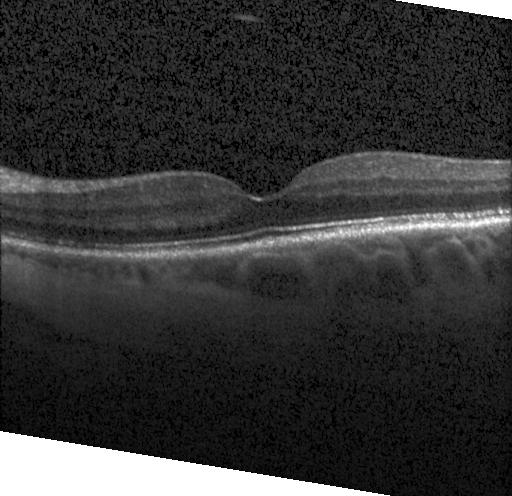

Retinal OCT B-scan · Heidelberg Spectralis OCT system — Assessment: neither CNV, DME, nor drusen.